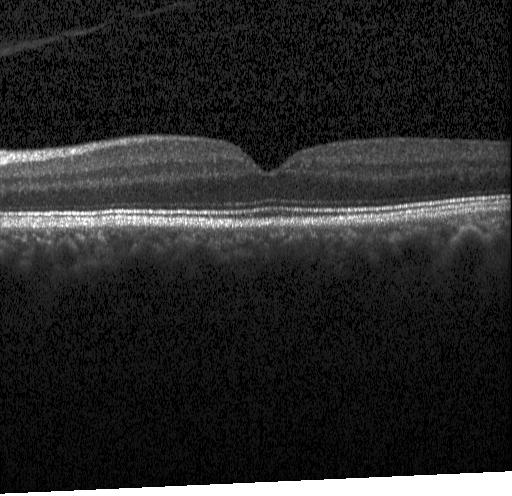

OCT line scan; through the macula; SD-OCT; instrument: Heidelberg Spectralis — Impression: no CNV, no DME, and no drusen.